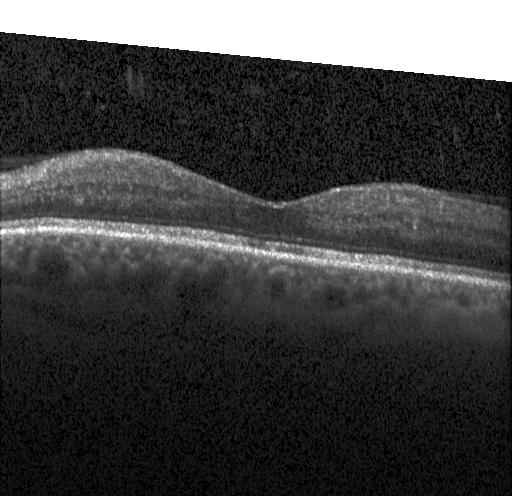
OCT line scan. Instrument: Heidelberg Spectralis. Diagnosis: no CNV, DME, or drusen.